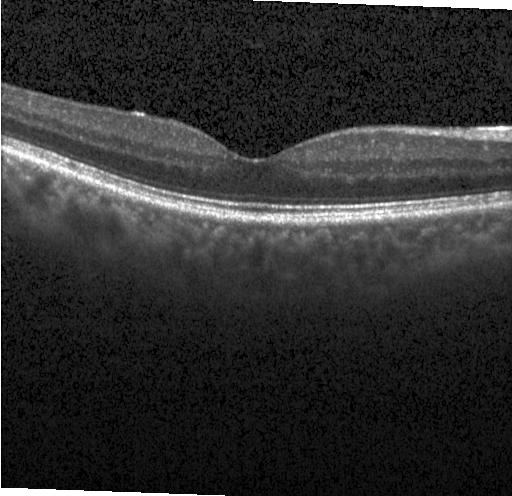 Fovea-centered. Spectral-domain OCT. Optical coherence tomography B-scan.
Macular OCT: no CNV, no DME, and no drusen.